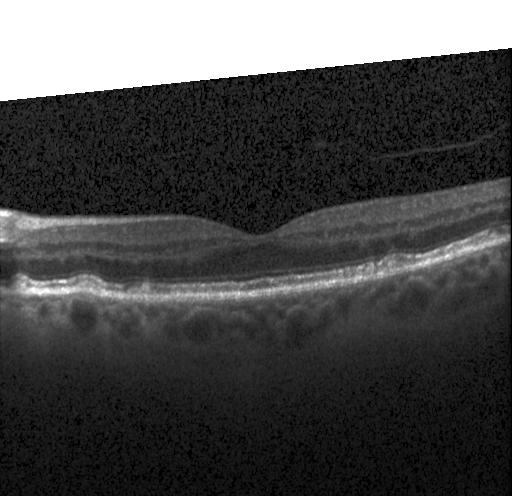 Dx: drusen.